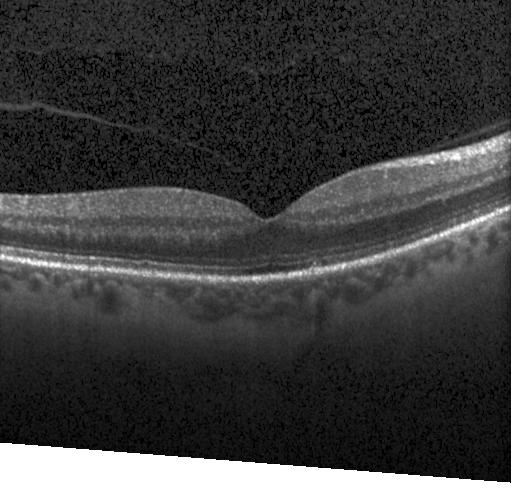

Retinal OCT cross-section showing neither CNV, DME, nor drusen.